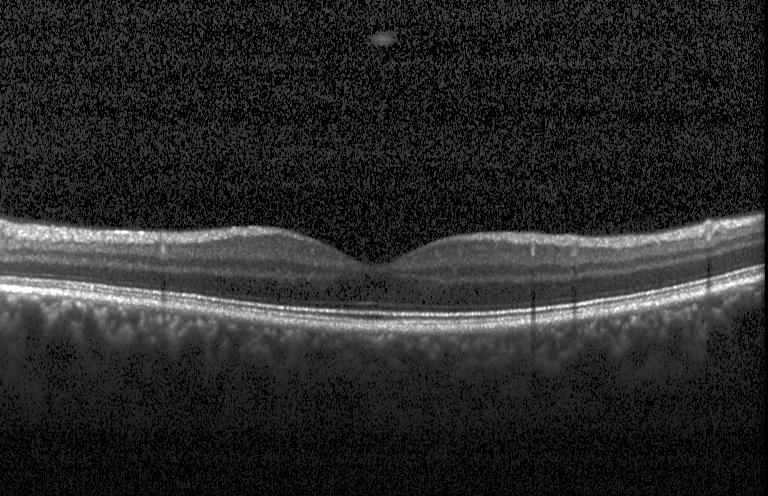
OCT finding: neither choroidal neovascularization, diabetic macular edema, nor drusen.